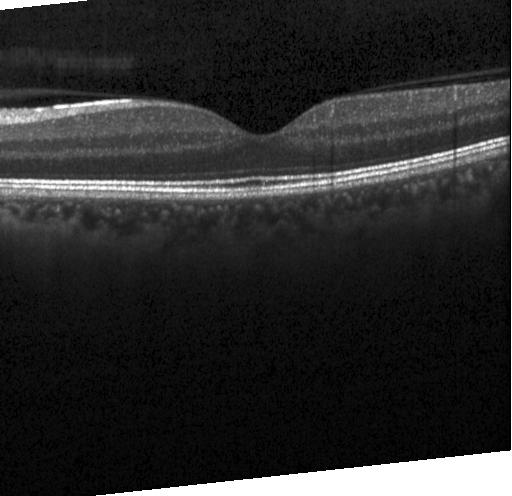 OCT finding: no choroidal neovascularization, diabetic macular edema, or drusen.